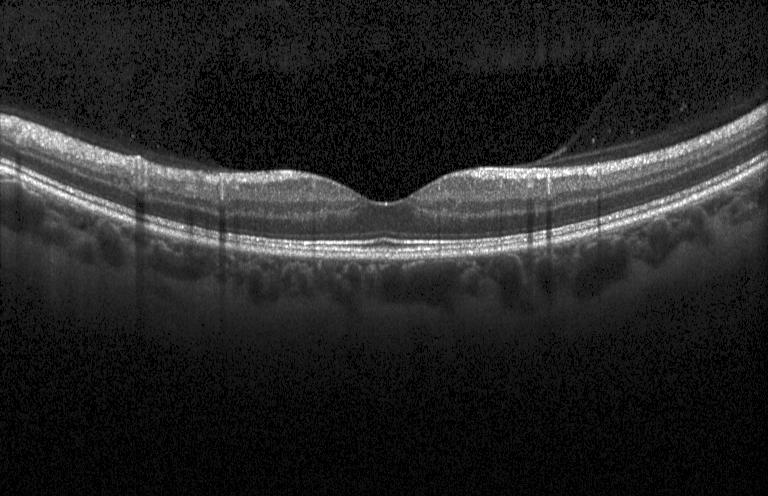

Instrument: Heidelberg Spectralis; retinal OCT B-scan
Finding: neither CNV, DME, nor drusen.